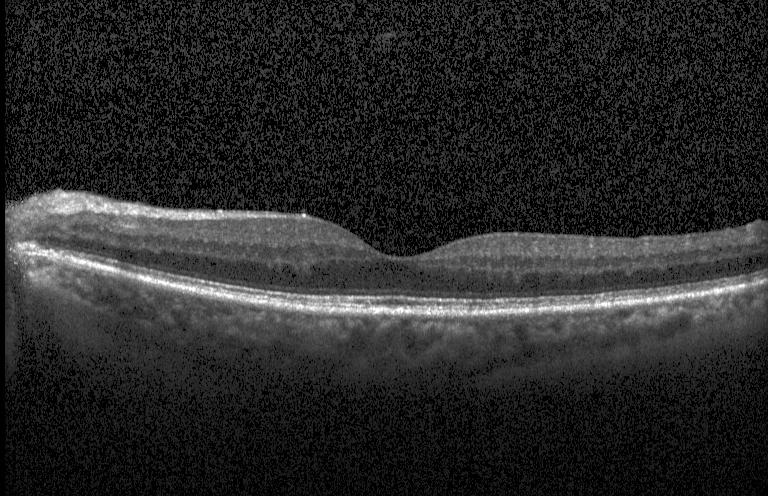 Impression: no CNV, no DME, and no drusen.